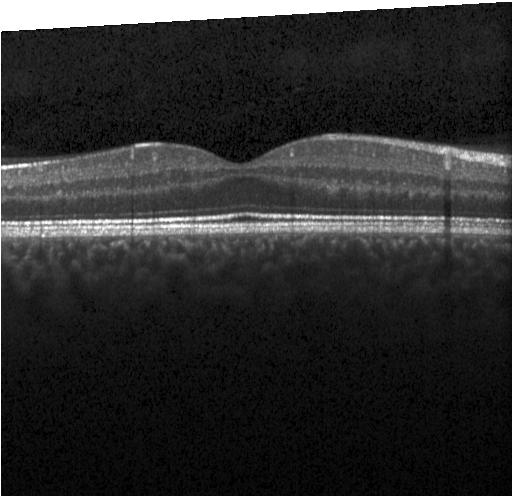 OCT line scan; spectral-domain OCT — Neither choroidal neovascularization, diabetic macular edema, nor drusen.